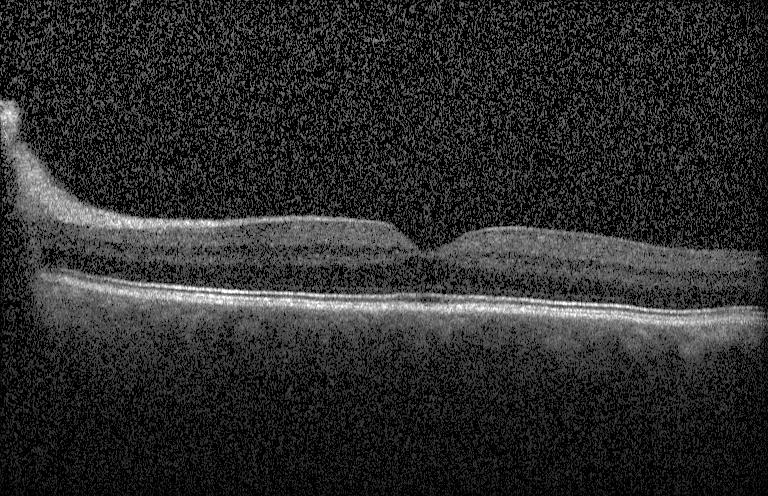
Impression: neither CNV, DME, nor drusen.